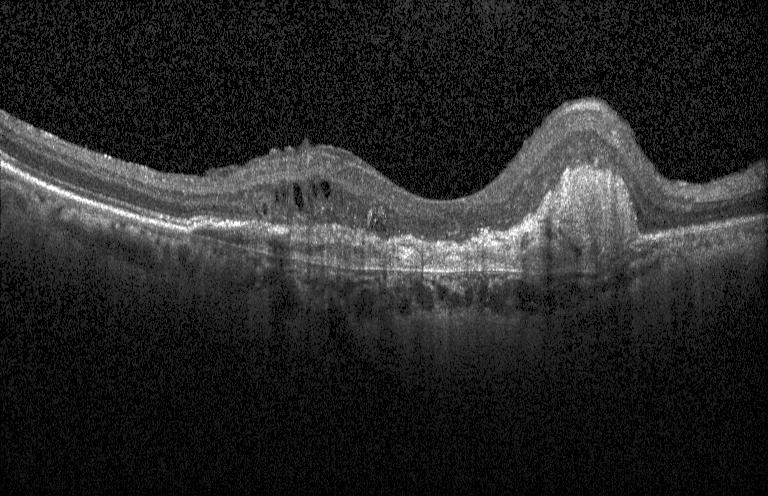

Retinal OCT cross-section.
This B-scan demonstrates CNV.